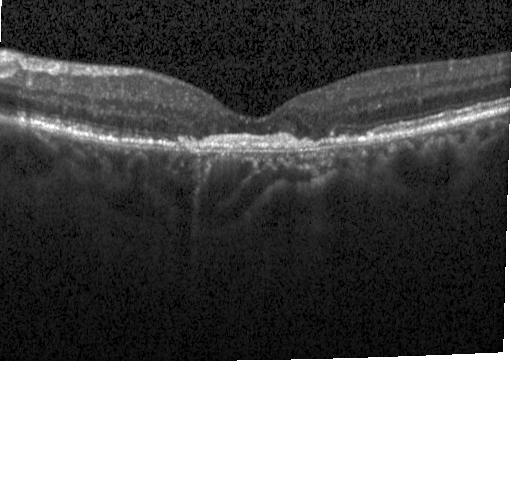 Optical coherence tomography scan — Choroidal neovascularization.